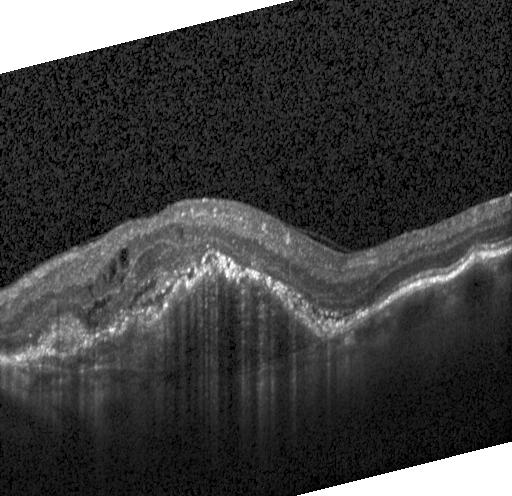 Impression: choroidal neovascularization.